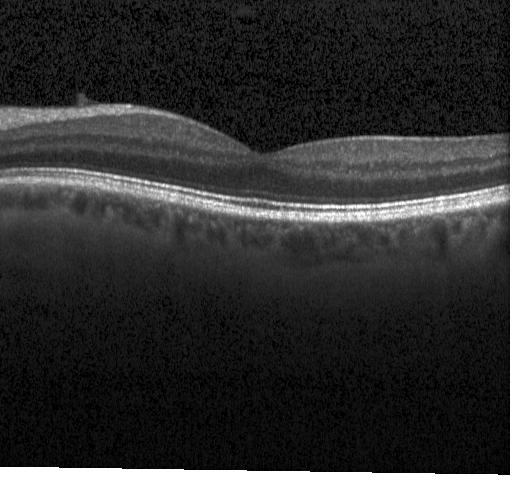 Heidelberg Spectralis · horizontal scan through the fovea · retinal OCT B-scan.
Assessment: no choroidal neovascularization, diabetic macular edema, or drusen.